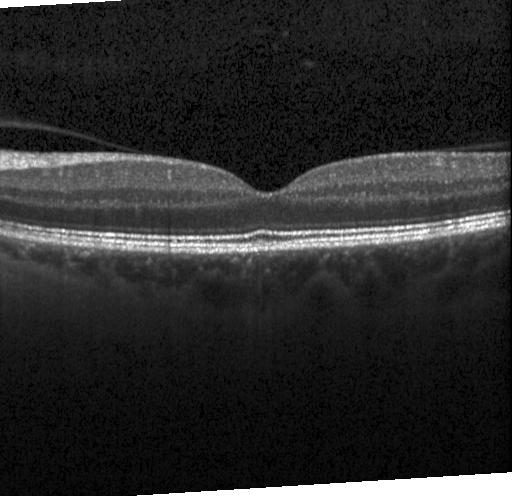
Optical coherence tomography scan.
The scan shows no CNV, no DME, and no drusen.